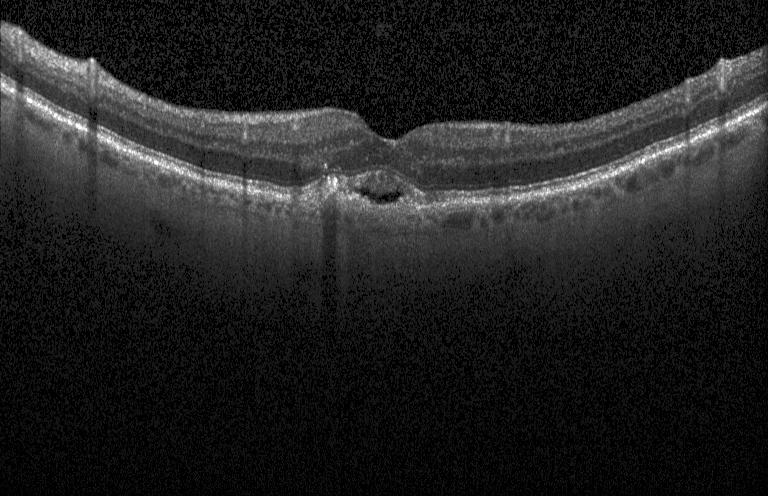 OCT line scan
Dx: choroidal neovascularization (CNV).